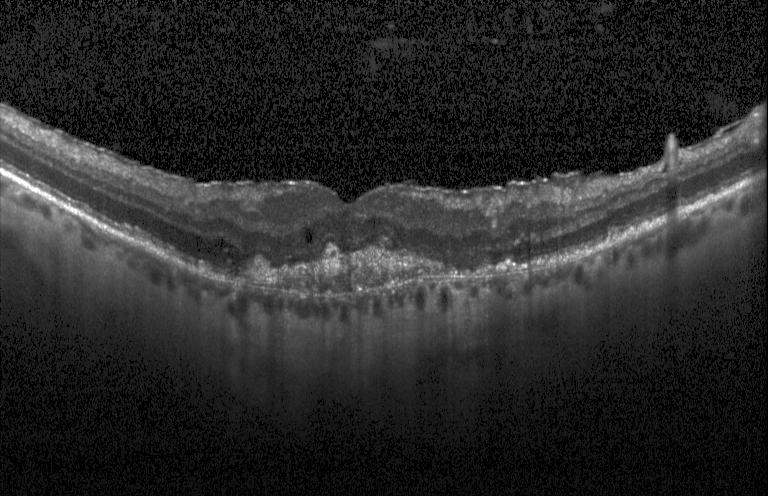

Retinal OCT cross-section — Macular OCT: choroidal neovascularization (CNV).